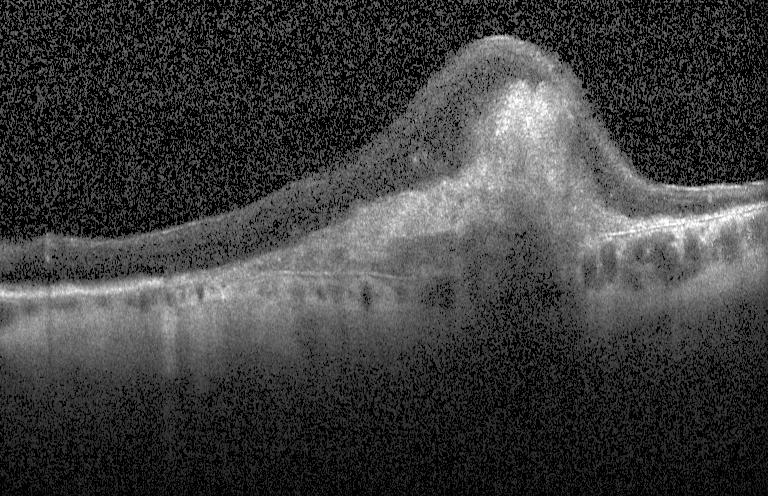
Spectral-domain optical coherence tomography, optical coherence tomography B-scan, fovea-centered — Impression: a choroidal neovascular membrane.